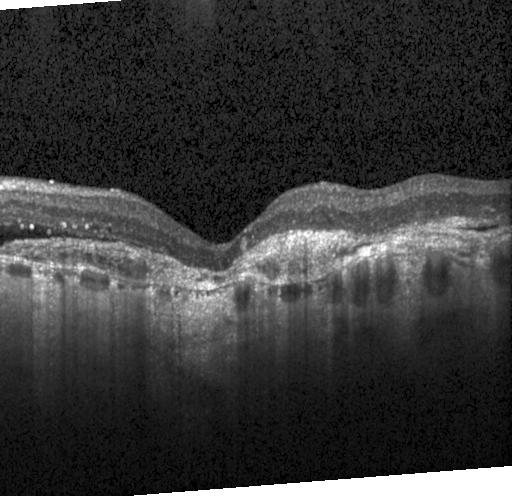 OCT B-scan — OCT finding: choroidal neovascularization.